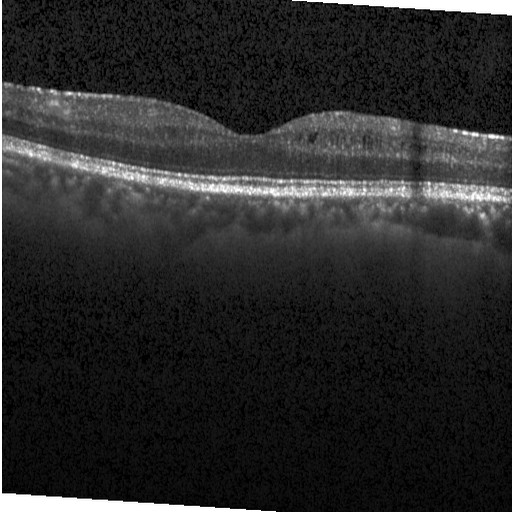

Acquired on a Heidelberg Spectralis. OCT B-scan.
Diabetic macular edema.